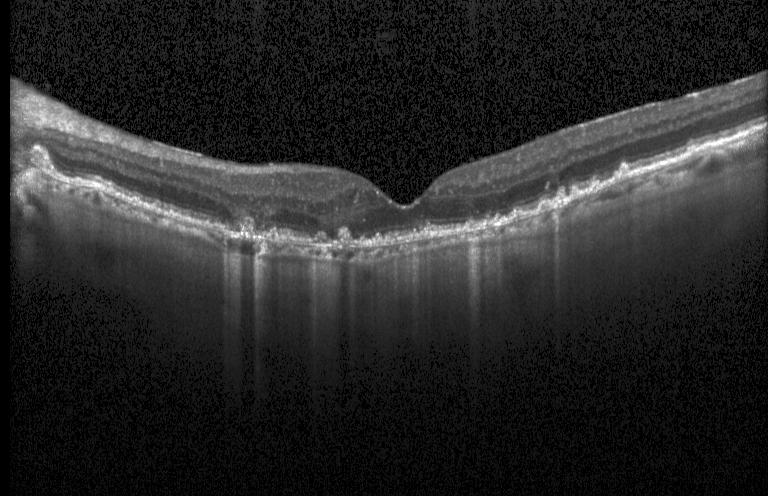

Spectral-domain OCT B-scan: a choroidal neovascular membrane.